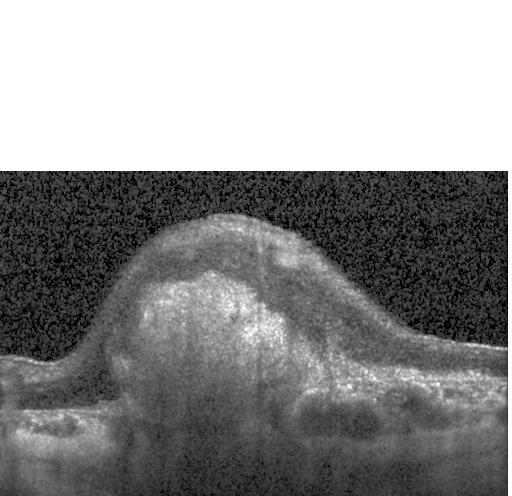 Dx: choroidal neovascularization.